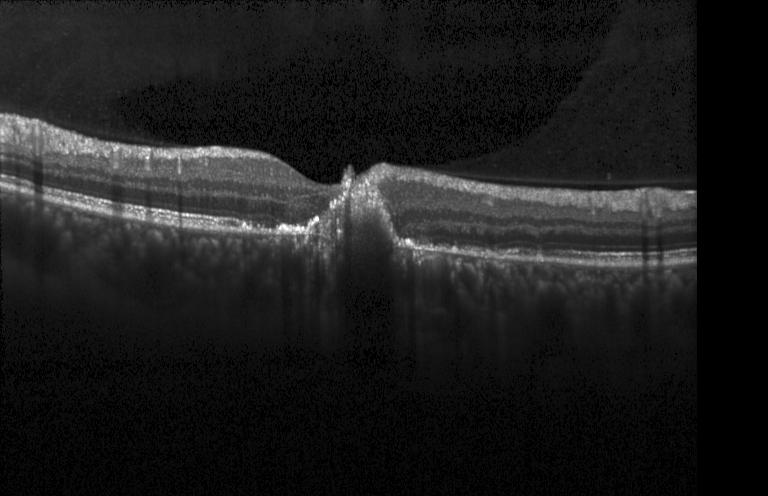 Diagnosis: CNV.